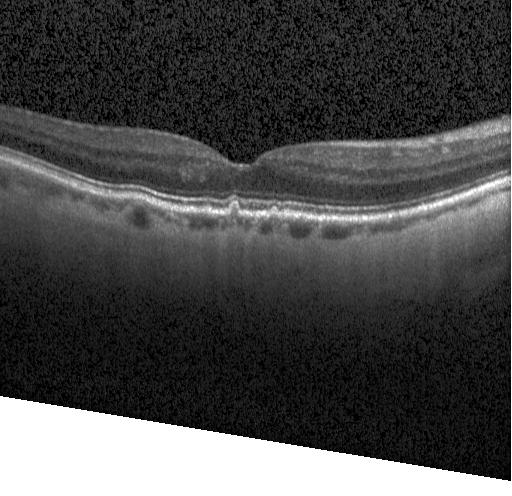

Retinal OCT cross-section, Heidelberg Spectralis OCT system, spectral-domain optical coherence tomography — Macular OCT: sub-RPE drusenoid deposits.